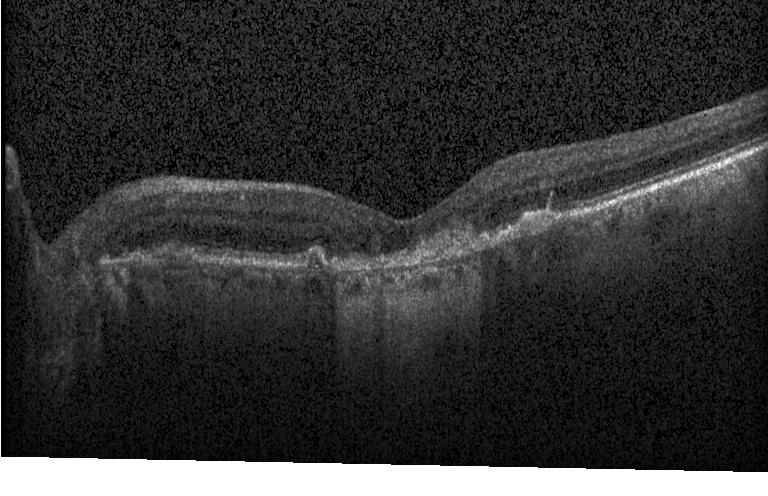 OCT line scan — Impression: CNV.